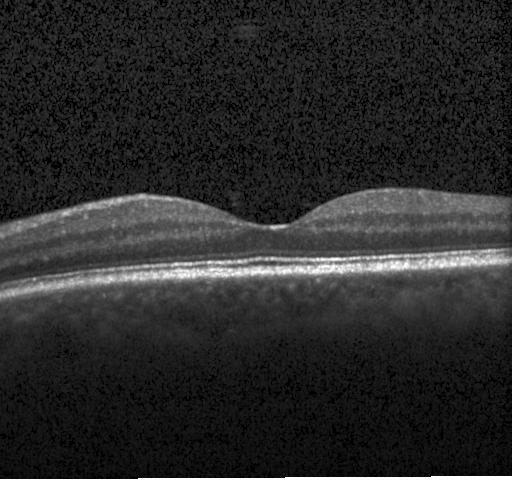 Retinal OCT cross-section showing no CNV, DME, or drusen.